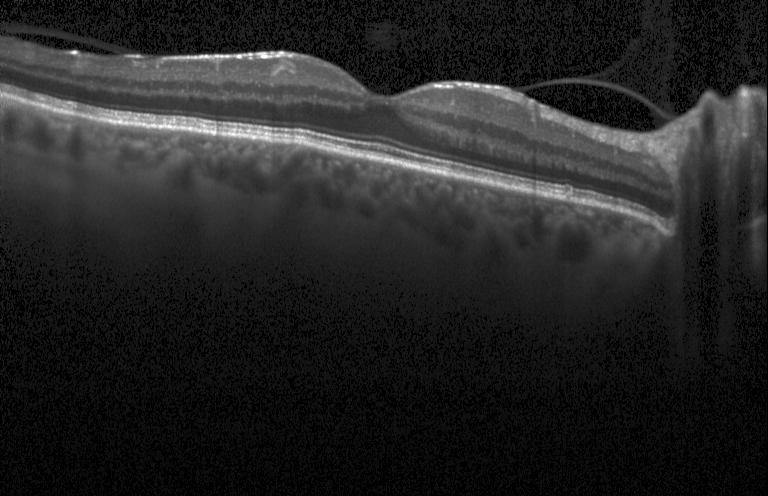
OCT B-scan · instrument: Heidelberg Spectralis — Finding: no CNV, DME, or drusen.